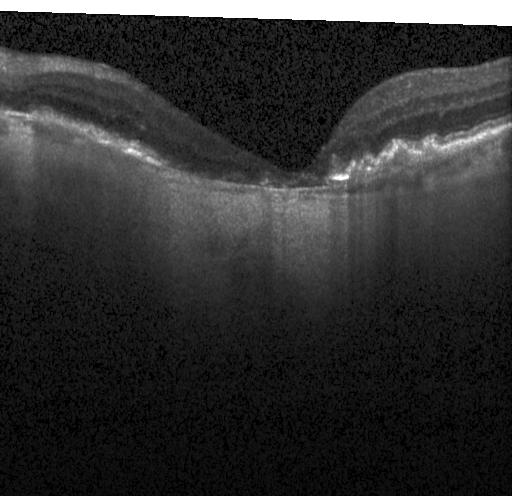 The scan shows choroidal neovascularization.